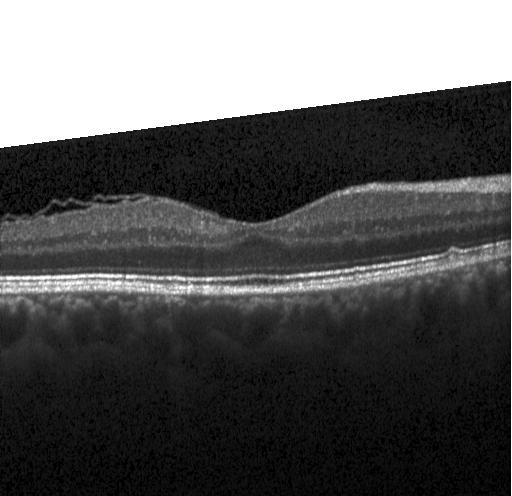 This B-scan demonstrates drusen.